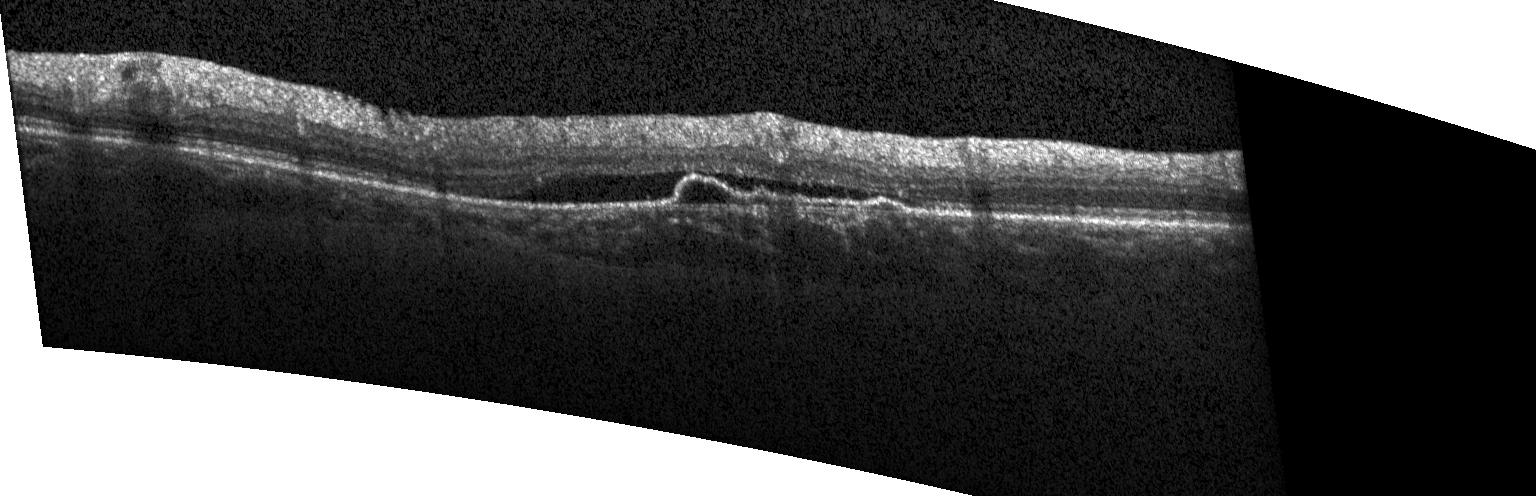

Fovea-centered, Heidelberg Spectralis OCT system, optical coherence tomography scan.
A choroidal neovascular membrane.